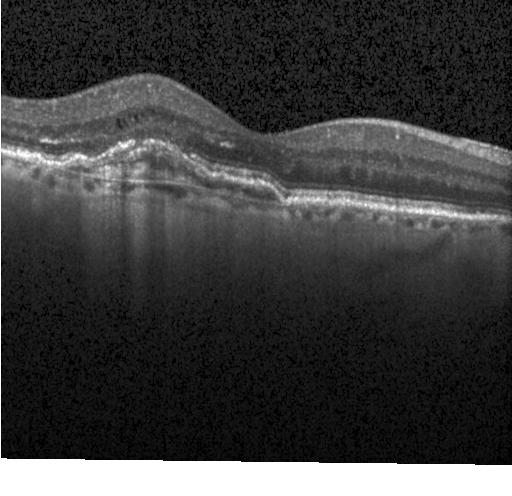

Spectral-domain OCT, retinal OCT B-scan, Heidelberg Spectralis — Impression: CNV.